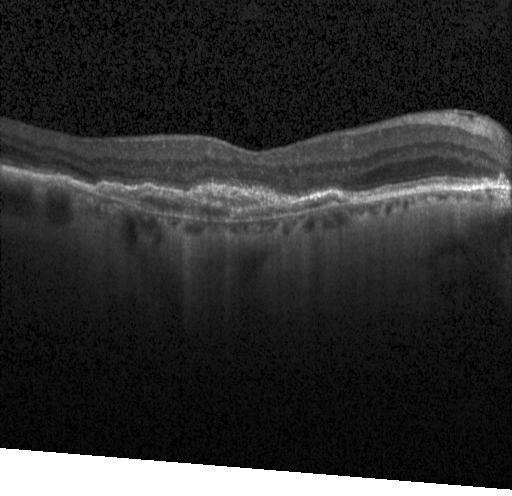
Macular OCT: a choroidal neovascular membrane.